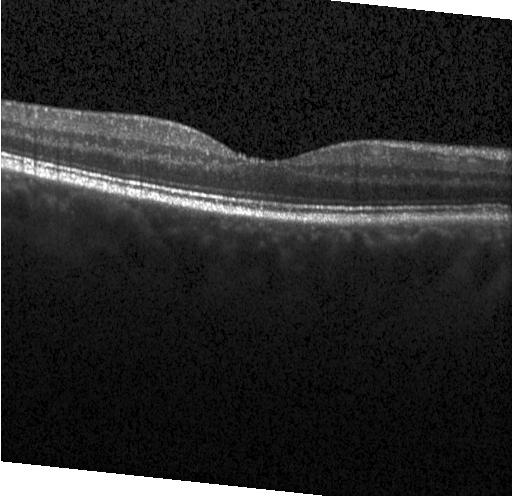 Spectral-domain optical coherence tomography · optical coherence tomography scan.
Impression: no evidence of choroidal neovascularization, diabetic macular edema, or drusen.